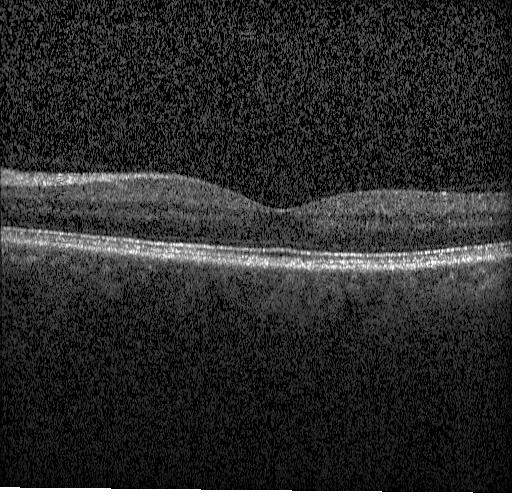

OCT line scan, spectral-domain OCT — This B-scan demonstrates no choroidal neovascularization, no diabetic macular edema, and no drusen.